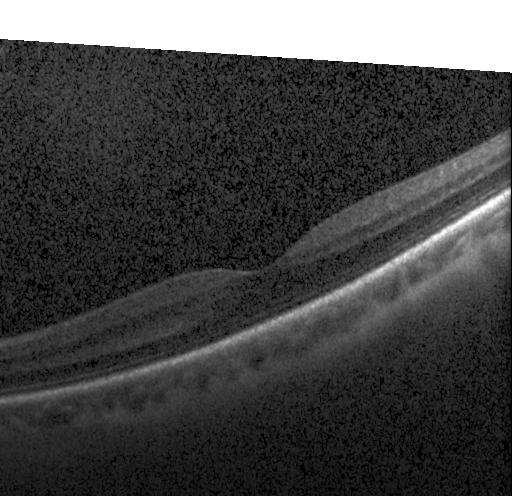
Fovea-centered, OCT B-scan, SD-OCT
Finding: neither choroidal neovascularization, diabetic macular edema, nor drusen.